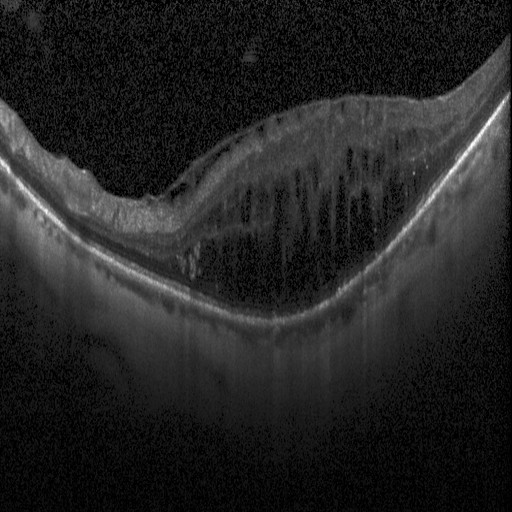
This B-scan demonstrates diabetic macular edema.